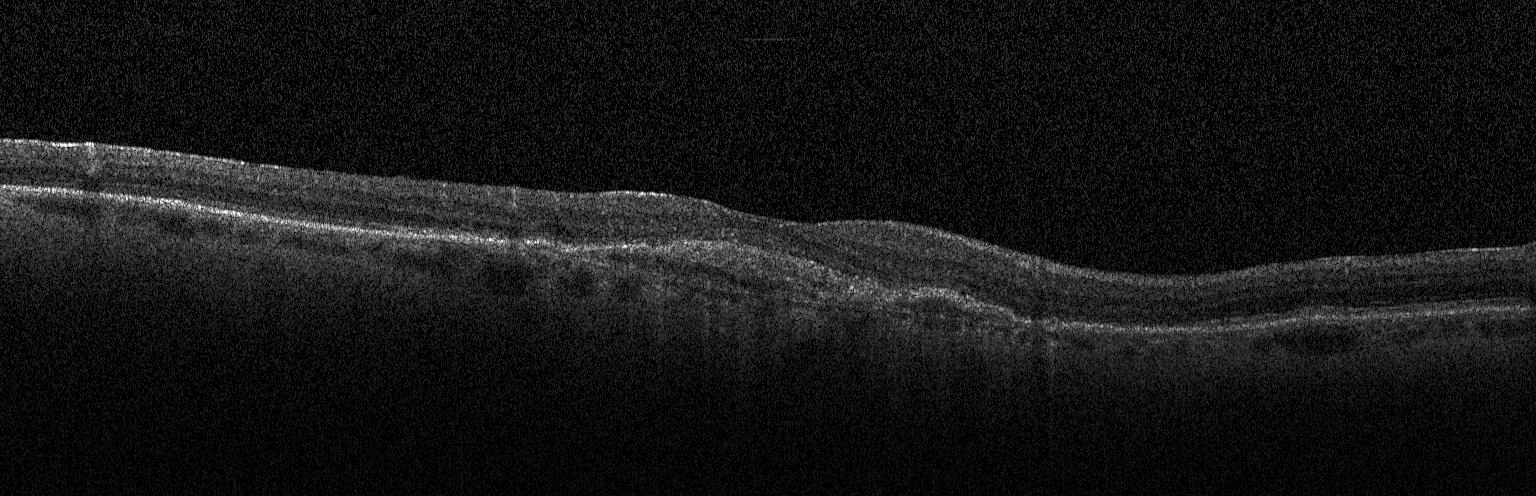
Spectral-domain OCT, OCT B-scan. Choroidal neovascularization (CNV).